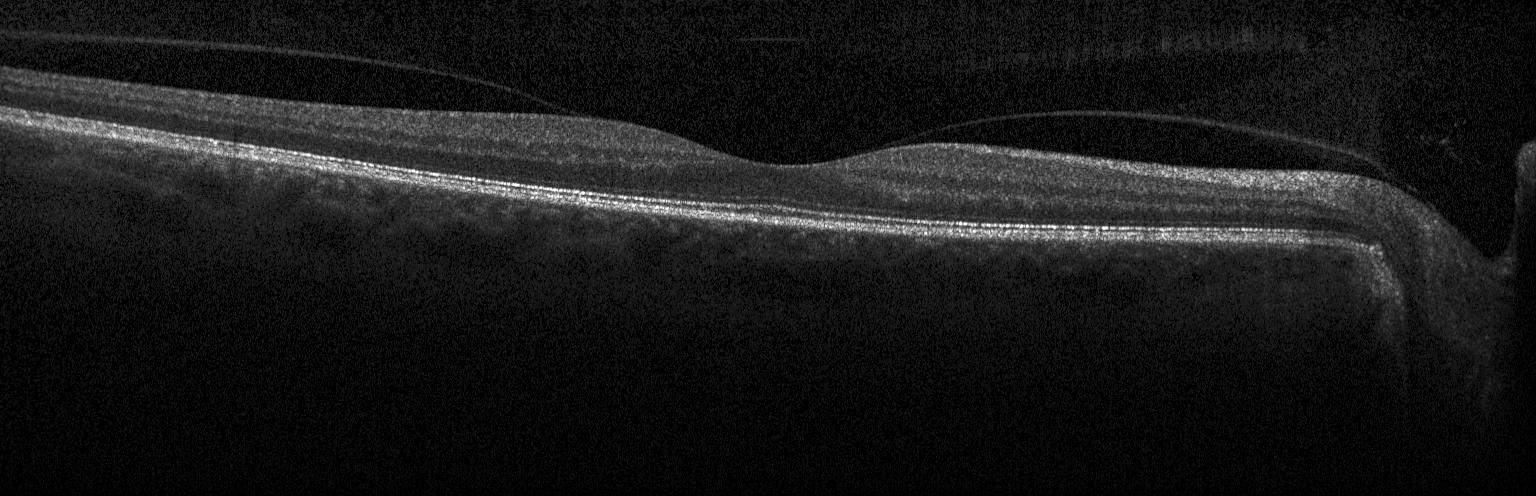 Horizontal scan through the fovea. Retinal OCT B-scan. Impression: neither choroidal neovascularization, diabetic macular edema, nor drusen.